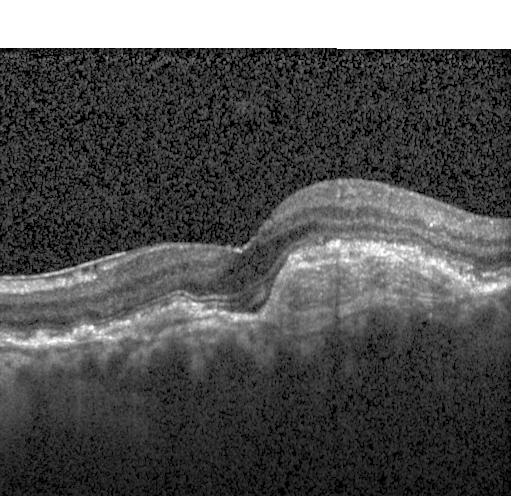

Spectral-domain OCT · optical coherence tomography B-scan · macular scan — Macular OCT: choroidal neovascularization.